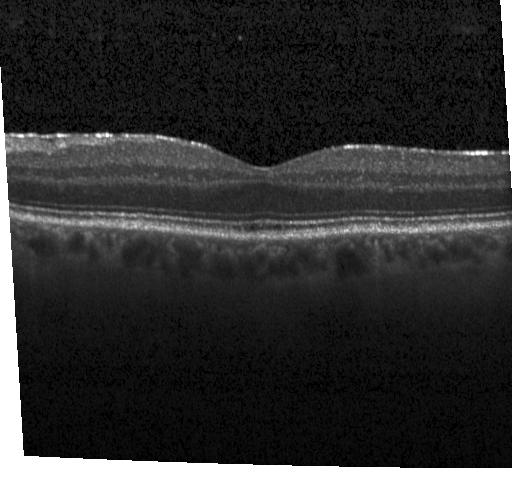
Impression: no evidence of choroidal neovascularization, diabetic macular edema, or drusen.